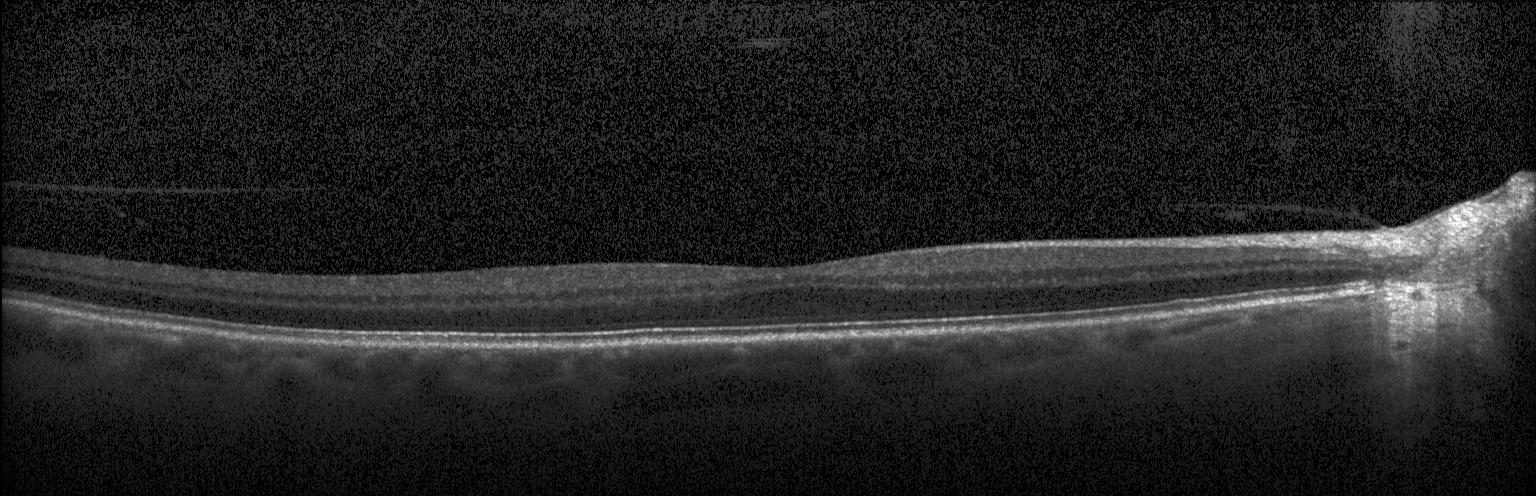
Macular scan, SD-OCT, retinal OCT B-scan — Impression: no CNV, DME, or drusen.